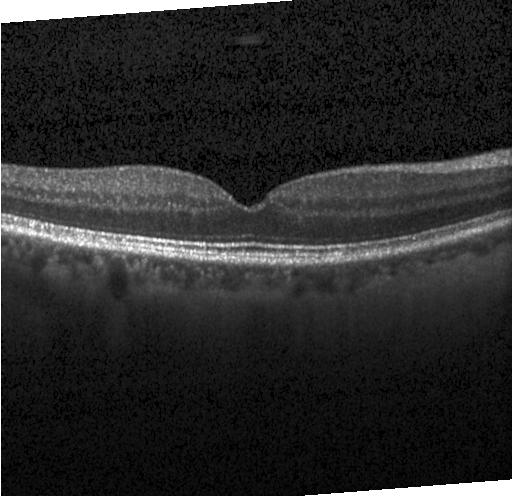 Macular scan, OCT B-scan, spectral-domain OCT, instrument: Heidelberg Spectralis. Diagnosis: no CNV, DME, or drusen.